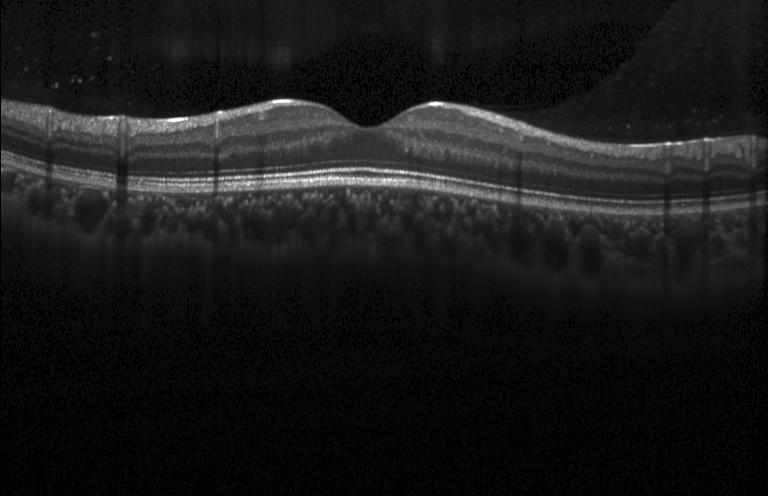 OCT scan showing no choroidal neovascularization, no diabetic macular edema, and no drusen.